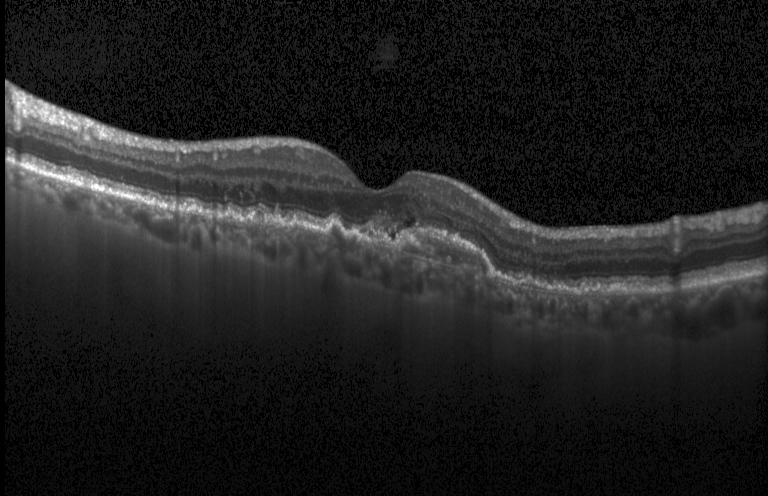 Diagnosis: a choroidal neovascular membrane.